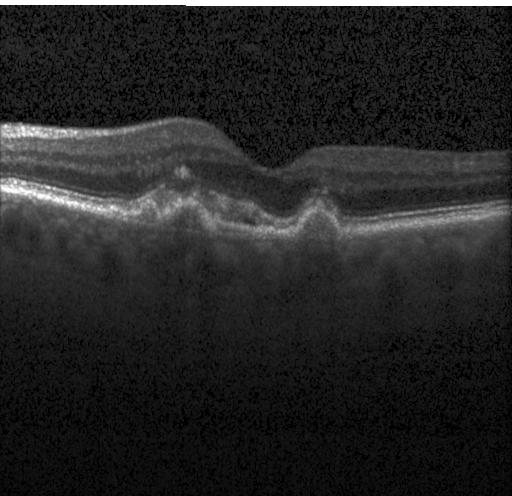

Impression: choroidal neovascularization.